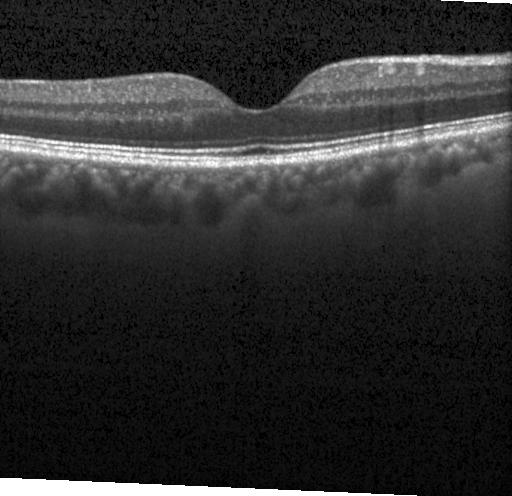

Macular scan; acquired on a Heidelberg Spectralis; OCT B-scan — Impression: no choroidal neovascularization, no diabetic macular edema, and no drusen.